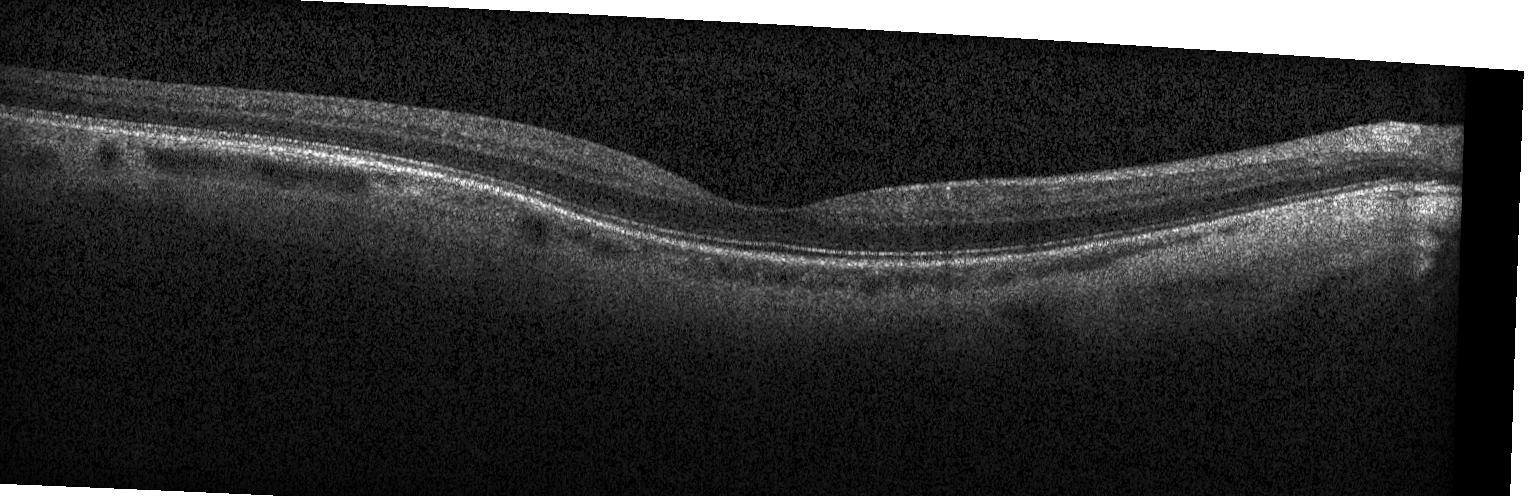 Finding: no evidence of choroidal neovascularization, diabetic macular edema, or drusen.